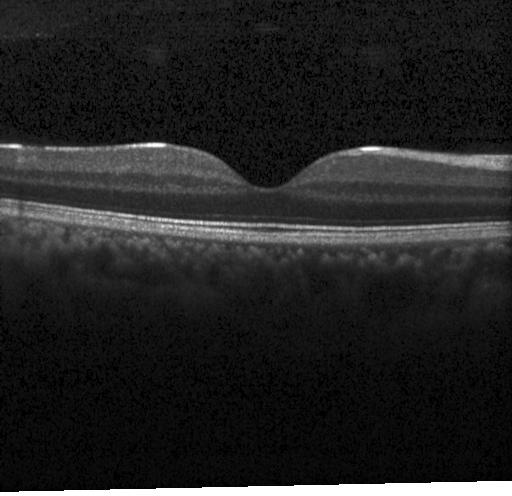 Optical coherence tomography scan, through the macula
OCT finding: no evidence of choroidal neovascularization, diabetic macular edema, or drusen.